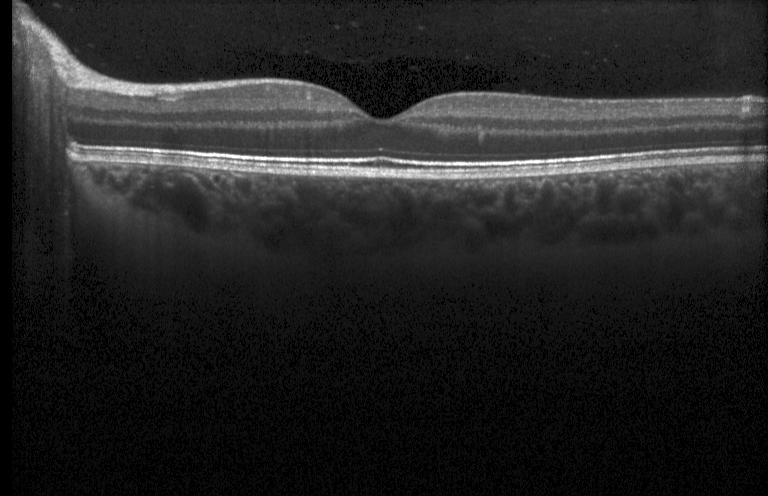
SD-OCT. Optical coherence tomography scan.
Finding: no choroidal neovascularization, no diabetic macular edema, and no drusen.